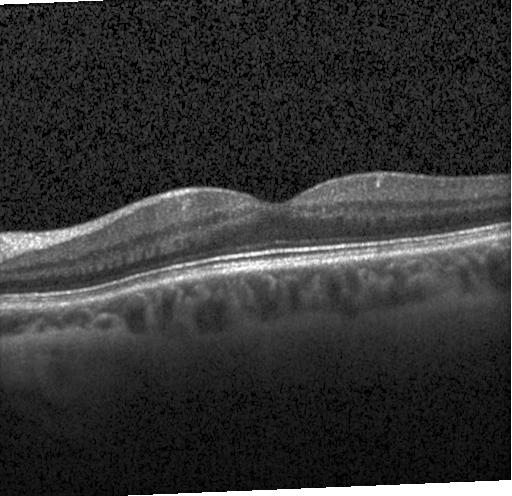 Retinal OCT B-scan.
Impression: no choroidal neovascularization, diabetic macular edema, or drusen.